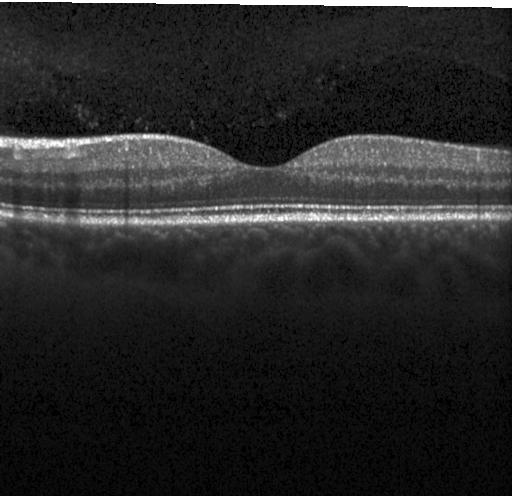
Optical coherence tomography scan.
Diagnosis: no choroidal neovascularization, diabetic macular edema, or drusen.